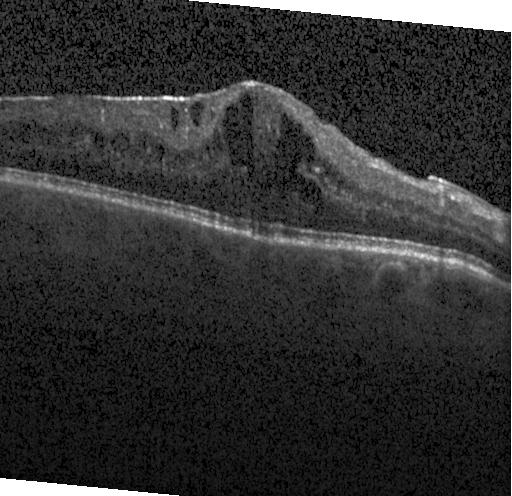 OCT finding: diabetic macular edema (DME).